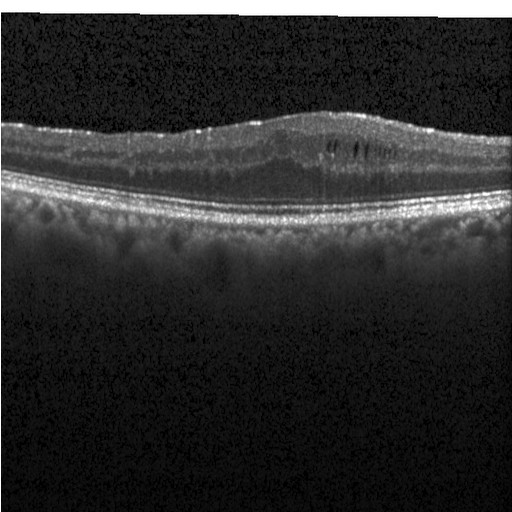
Retinal OCT cross-section. Finding: DME.